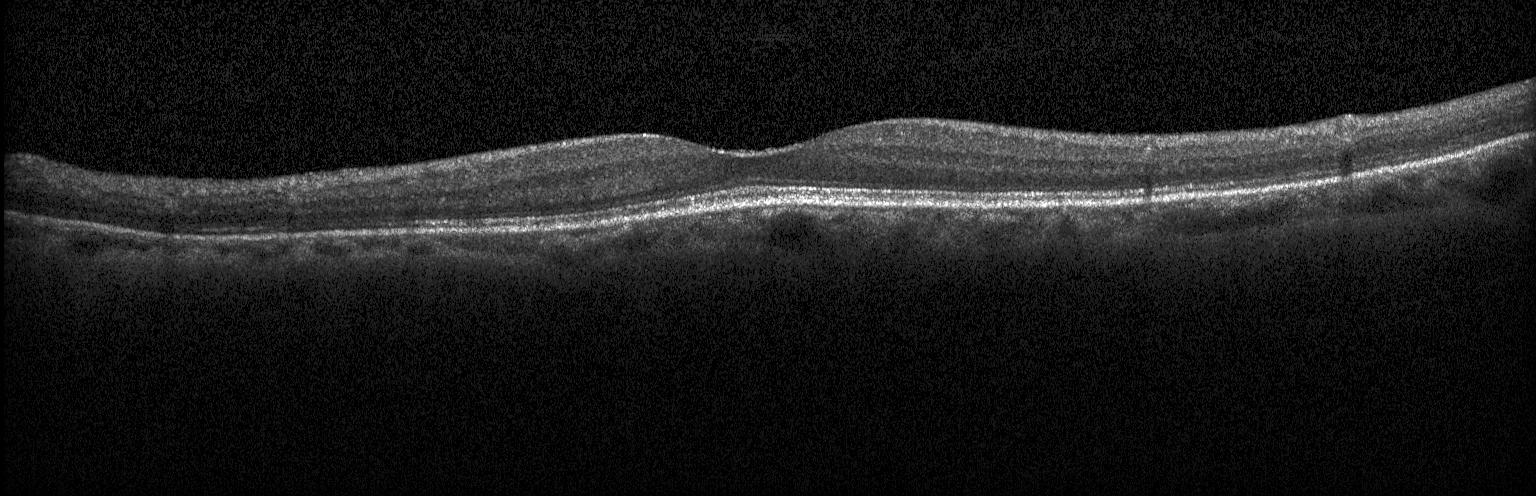
Finding: no choroidal neovascularization, diabetic macular edema, or drusen.